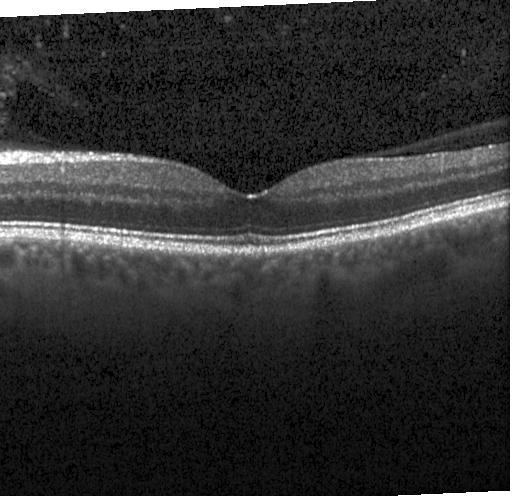
Fovea-centered. Optical coherence tomography scan. Spectral-domain OCT. Heidelberg Spectralis OCT system.
Assessment: no choroidal neovascularization, no diabetic macular edema, and no drusen.